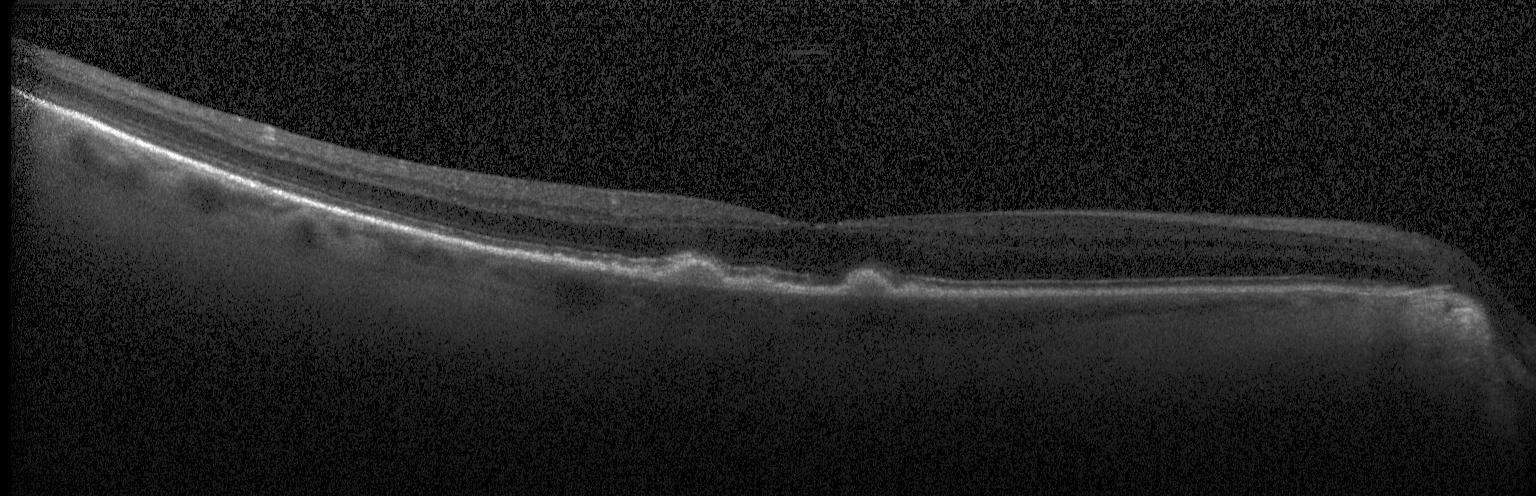 OCT finding: multiple drusen.